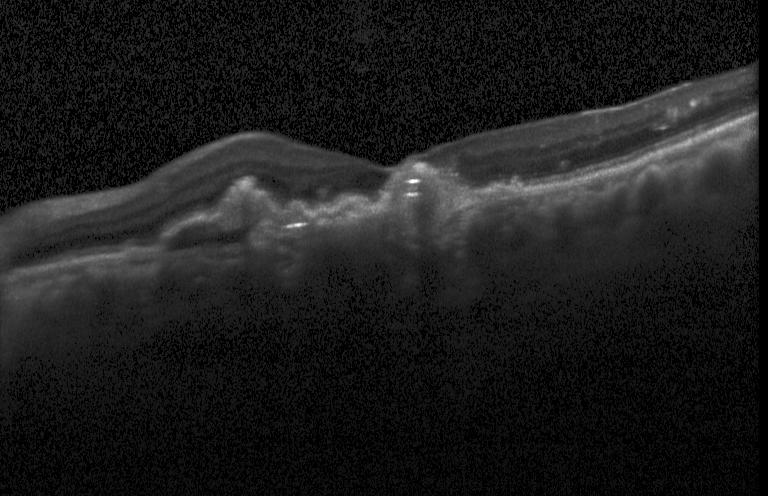

Spectral-domain OCT · acquired on a Heidelberg Spectralis · OCT line scan · horizontal scan through the fovea — Macular OCT: CNV.